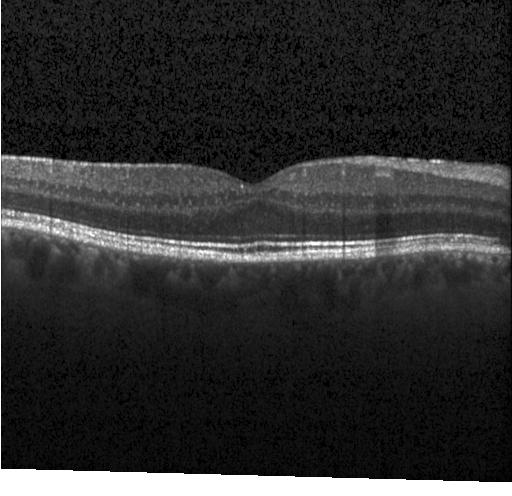

No choroidal neovascularization, no diabetic macular edema, and no drusen.